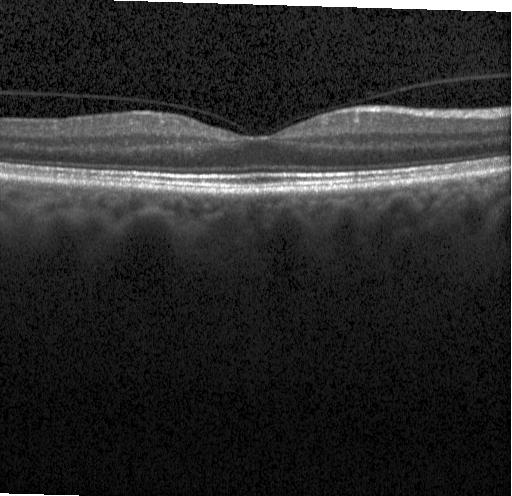

Optical coherence tomography B-scan, SD-OCT, Heidelberg Spectralis, macular scan. Impression: neither choroidal neovascularization, diabetic macular edema, nor drusen.